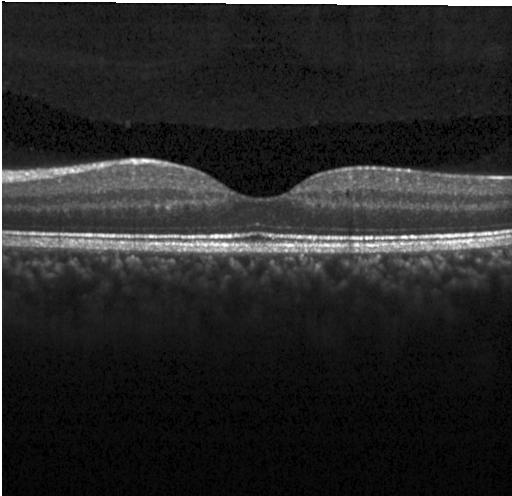

Optical coherence tomography B-scan — OCT finding: no evidence of choroidal neovascularization, diabetic macular edema, or drusen.